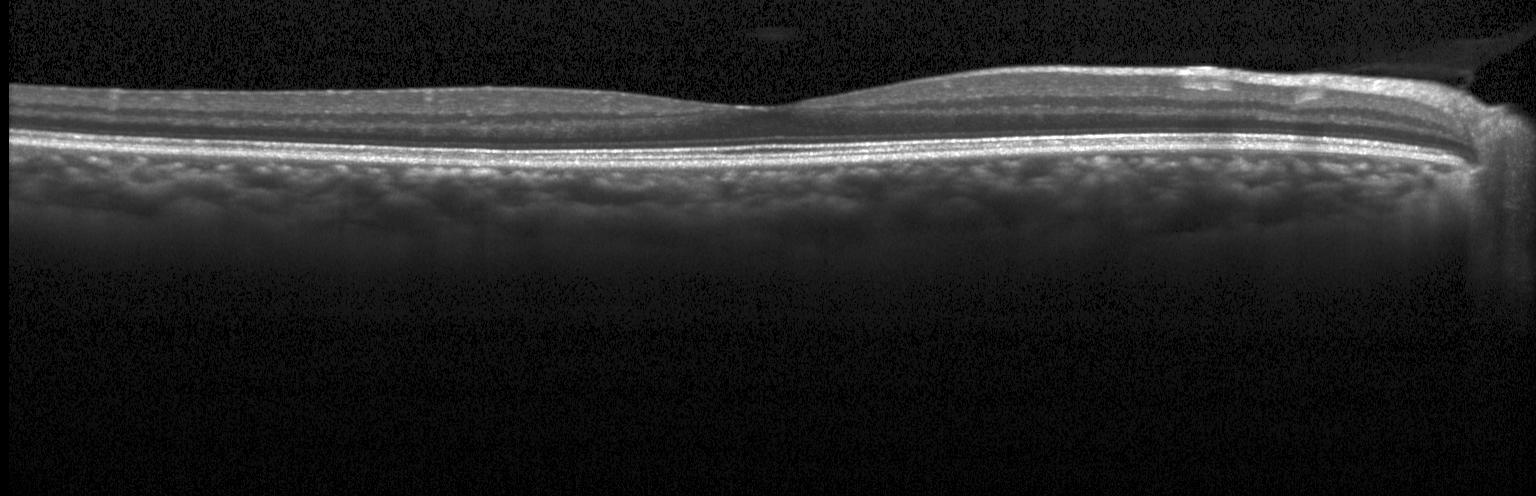

Centered on the fovea, acquired on a Heidelberg Spectralis, OCT line scan — This B-scan demonstrates no evidence of choroidal neovascularization, diabetic macular edema, or drusen.